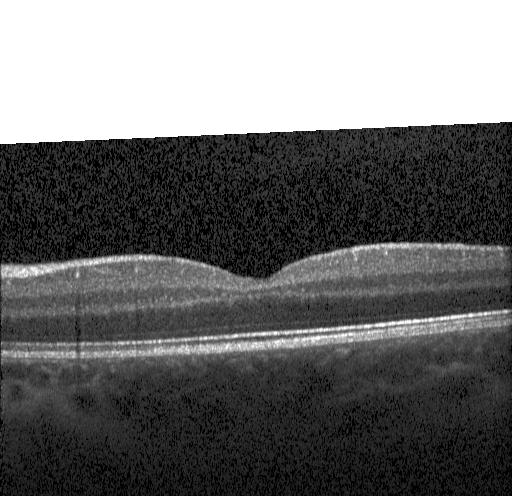

Assessment: neither choroidal neovascularization, diabetic macular edema, nor drusen.